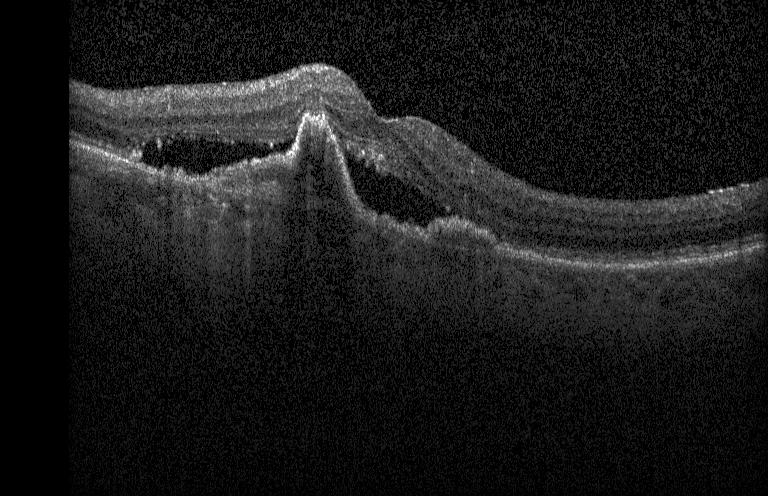
Macular OCT demonstrating choroidal neovascularization.